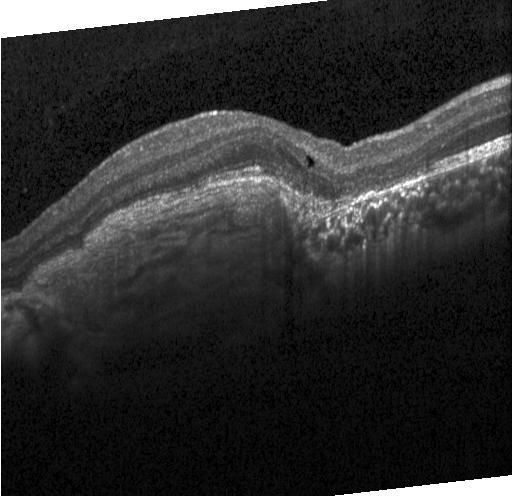 Optical coherence tomography scan · acquired on a Heidelberg Spectralis · macular scan
Finding: a choroidal neovascular membrane.